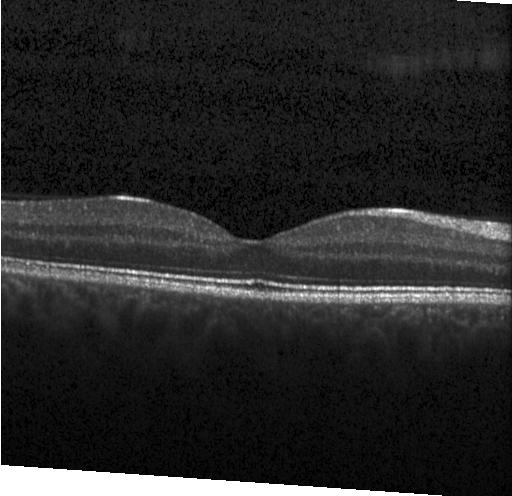
Impression: neither choroidal neovascularization, diabetic macular edema, nor drusen.